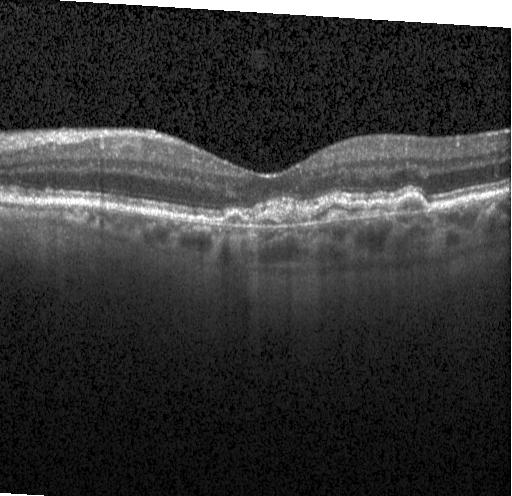 Spectral-domain OCT B-scan: CNV.